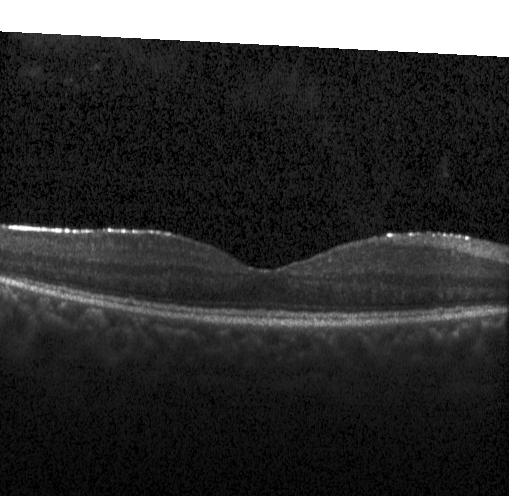

OCT B-scan.
This B-scan demonstrates no CNV, DME, or drusen.